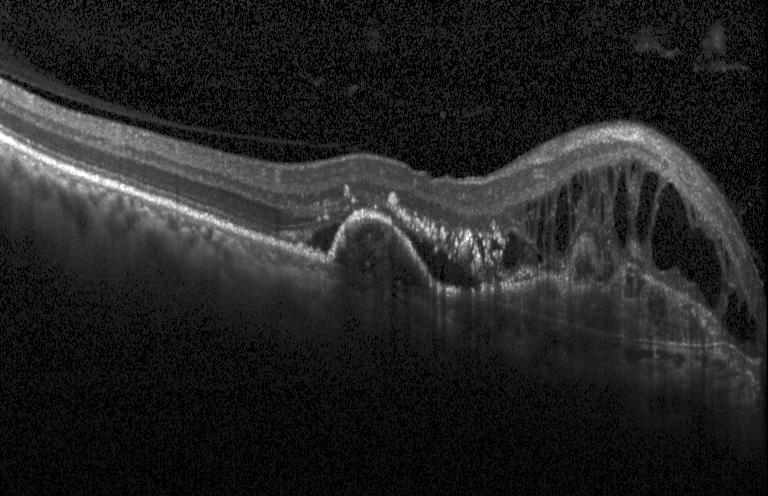
Spectral-domain OCT · optical coherence tomography scan.
Impression: a choroidal neovascular membrane.